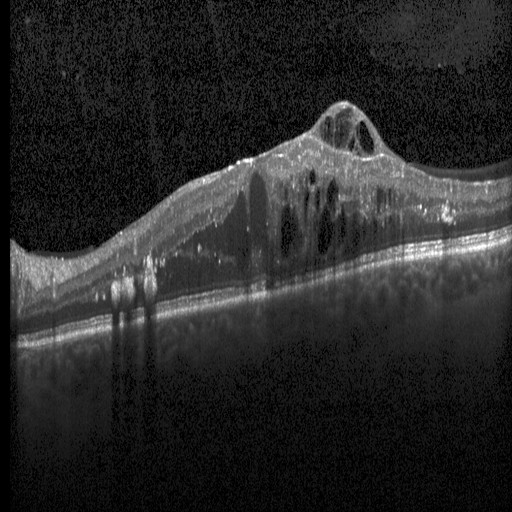
Retinal OCT B-scan
Finding: diabetic macular edema.